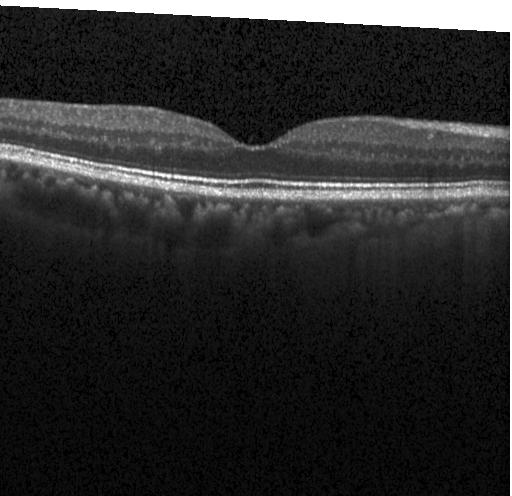 Acquired on a Heidelberg Spectralis, spectral-domain OCT, retinal OCT B-scan, fovea-centered.
OCT finding: no choroidal neovascularization, no diabetic macular edema, and no drusen.